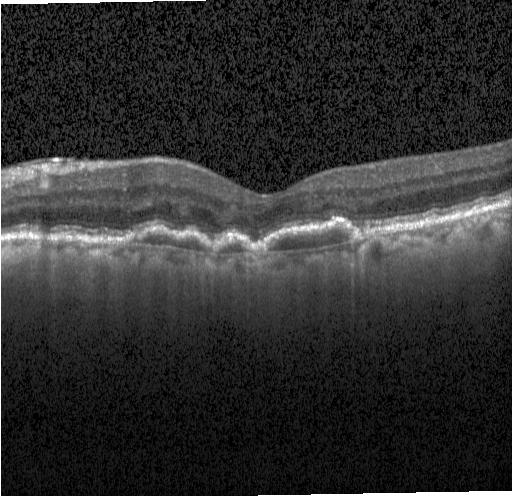 Through the macula; OCT B-scan; spectral-domain OCT; Heidelberg Spectralis OCT system
The scan shows a choroidal neovascular membrane.